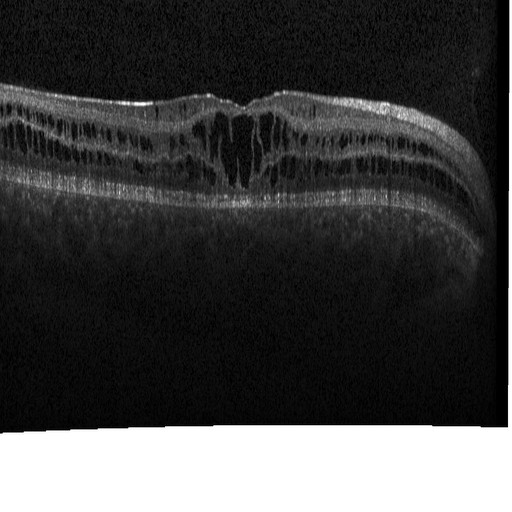 Assessment: DME.